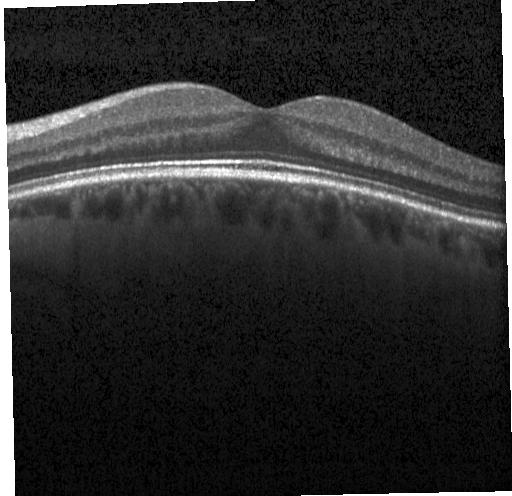 OCT scan showing no CNV, DME, or drusen.